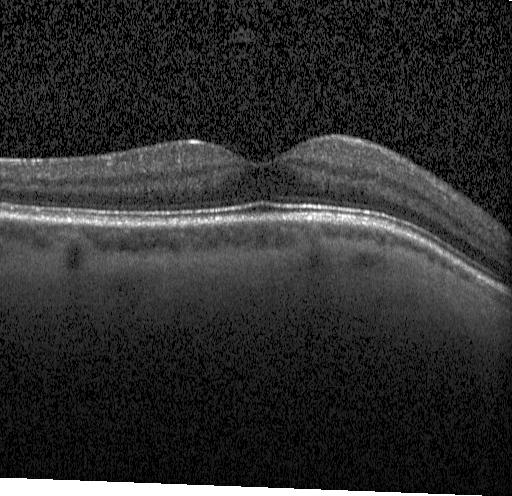

OCT scan showing neither CNV, DME, nor drusen.